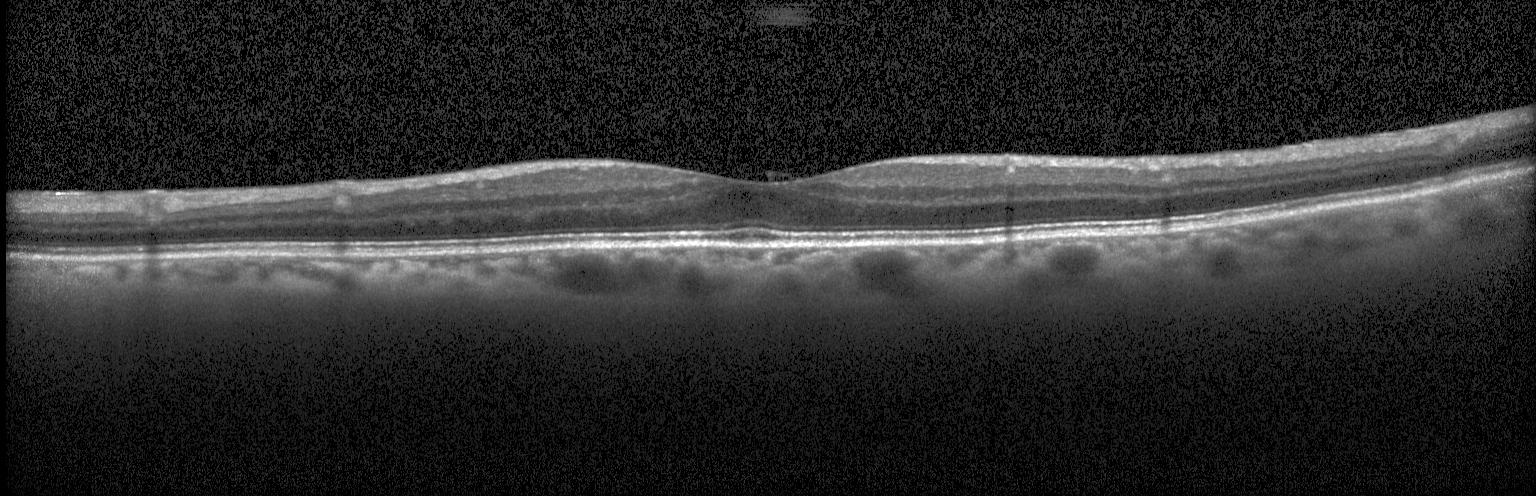
OCT line scan. Finding: no choroidal neovascularization, no diabetic macular edema, and no drusen.